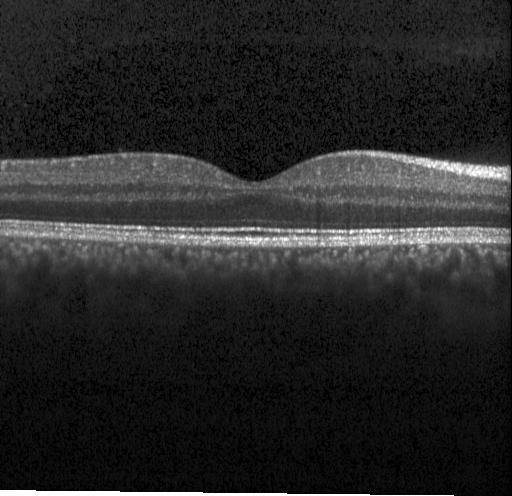

OCT line scan
This B-scan demonstrates no evidence of choroidal neovascularization, diabetic macular edema, or drusen.